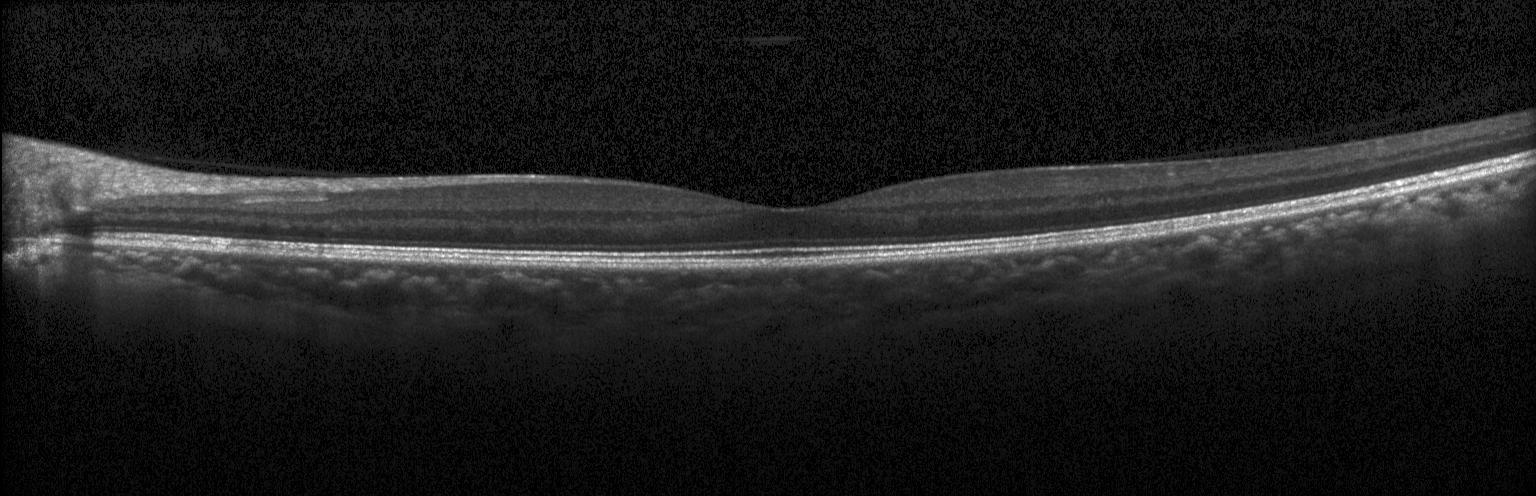 Retinal OCT B-scan, centered on the fovea, instrument: Heidelberg Spectralis, spectral-domain OCT. Finding: no choroidal neovascularization, no diabetic macular edema, and no drusen.